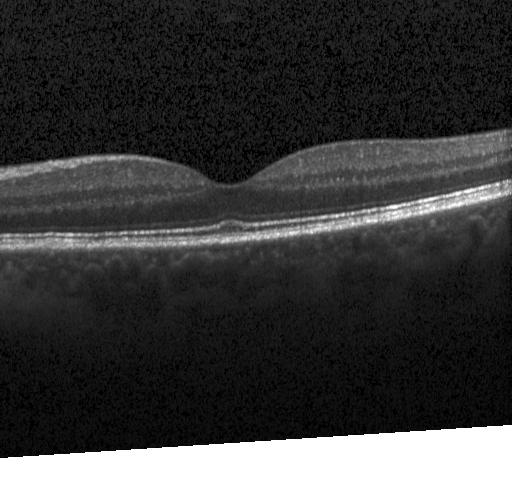 Instrument: Heidelberg Spectralis. OCT B-scan — Impression: no choroidal neovascularization, diabetic macular edema, or drusen.